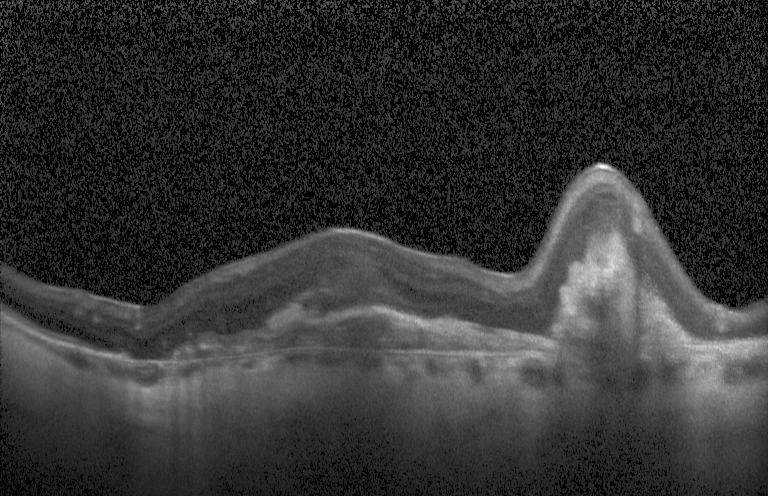

Optical coherence tomography B-scan. Impression: choroidal neovascularization (CNV).